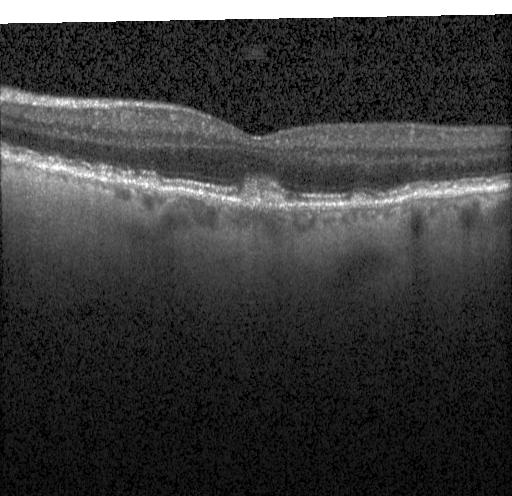

Horizontal scan through the fovea, OCT line scan, spectral-domain OCT. Impression: sub-RPE drusenoid deposits.